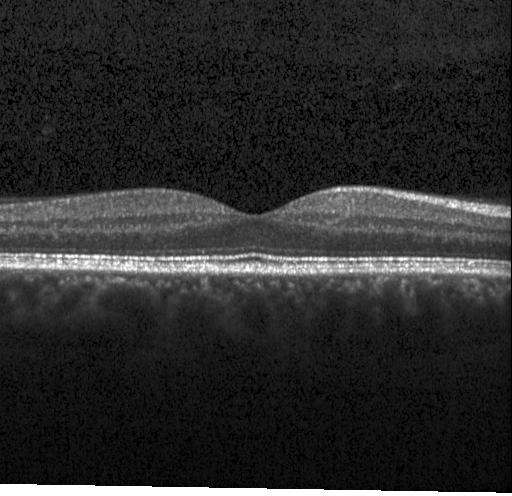

Spectral-domain OCT B-scan: no evidence of choroidal neovascularization, diabetic macular edema, or drusen.